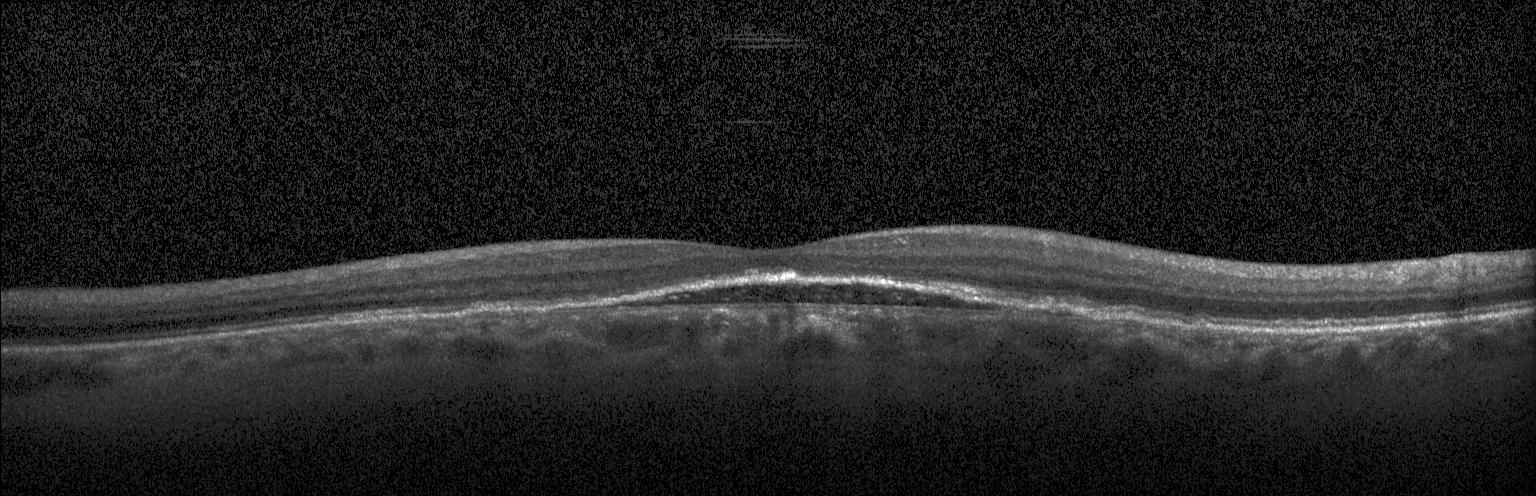 Instrument: Heidelberg Spectralis. Optical coherence tomography B-scan. Spectral-domain OCT. Macular scan. The scan shows choroidal neovascularization (CNV).